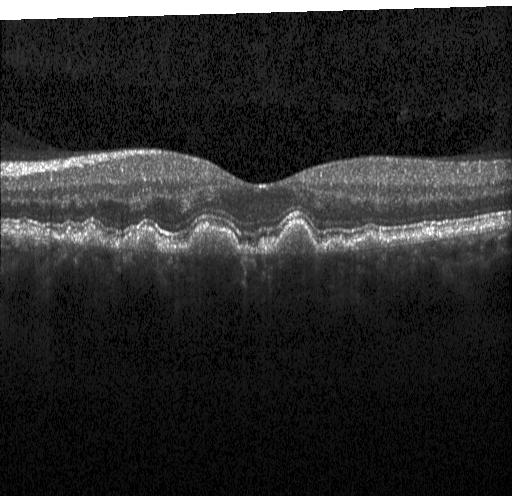 Dx: drusen.